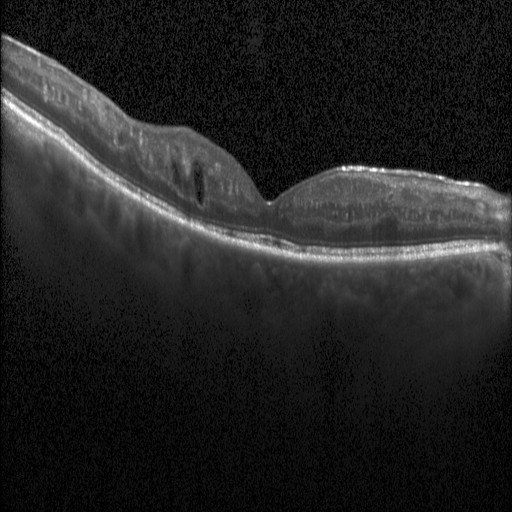

SD-OCT, retinal OCT B-scan
Diagnosis: diabetic macular edema (DME).